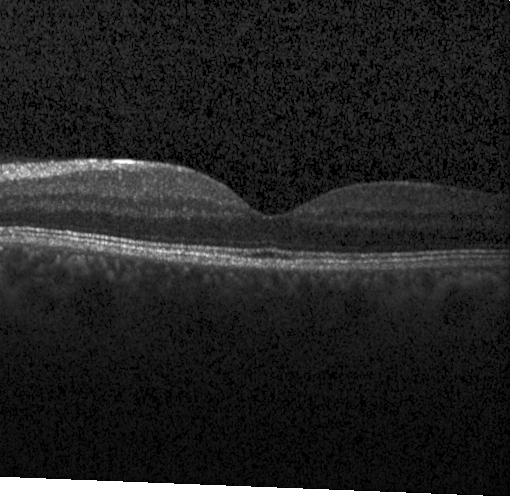

Optical coherence tomography scan. Impression: no CNV, DME, or drusen.